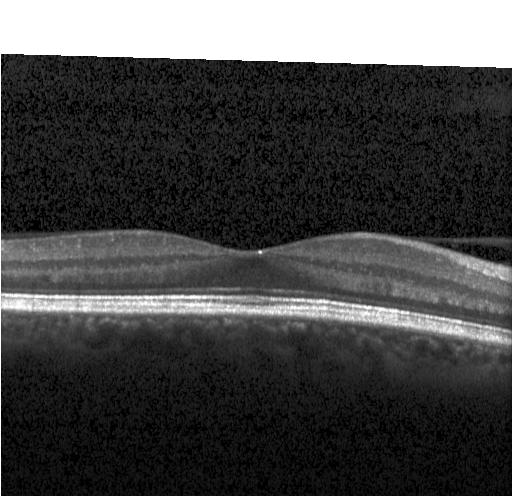 Optical coherence tomography scan. The scan shows no choroidal neovascularization, diabetic macular edema, or drusen.